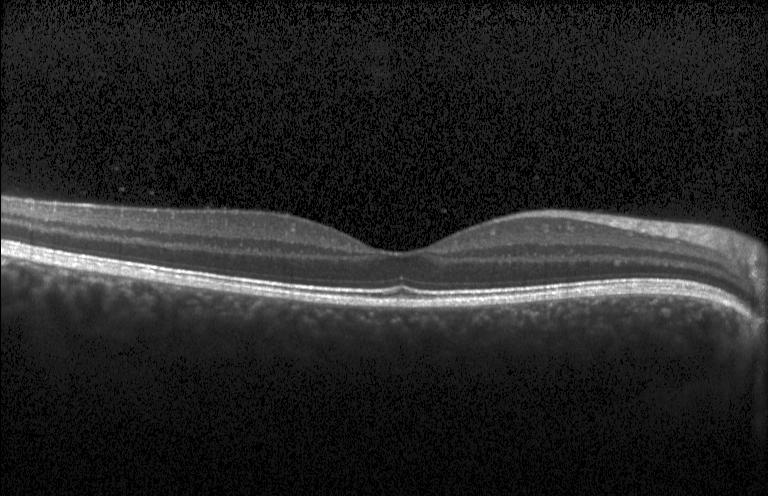

Dx: no choroidal neovascularization, no diabetic macular edema, and no drusen.